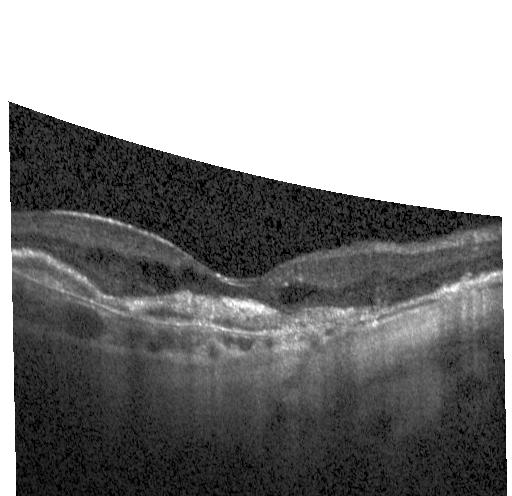 SD-OCT; macular scan; acquired on a Heidelberg Spectralis; retinal OCT cross-section.
Dx: a choroidal neovascular membrane.